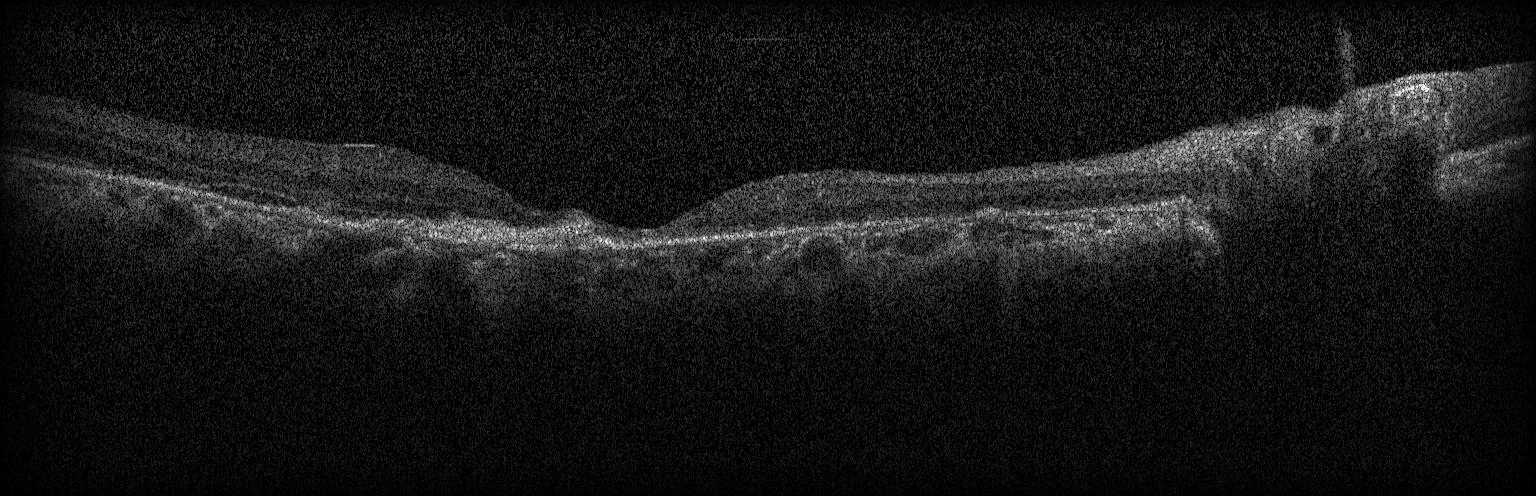

Spectral-domain optical coherence tomography · retinal OCT B-scan · Heidelberg Spectralis.
Macular OCT: a choroidal neovascular membrane.